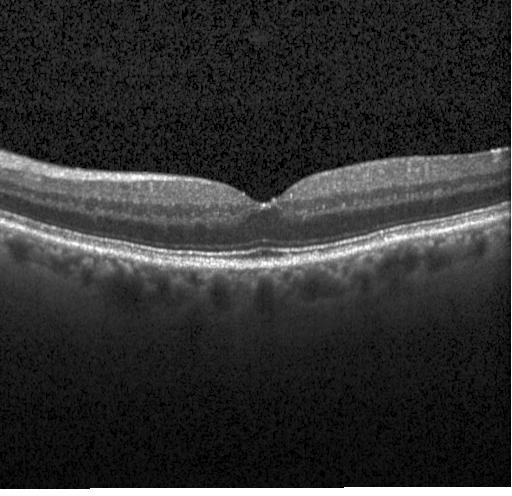 Impression: neither choroidal neovascularization, diabetic macular edema, nor drusen.